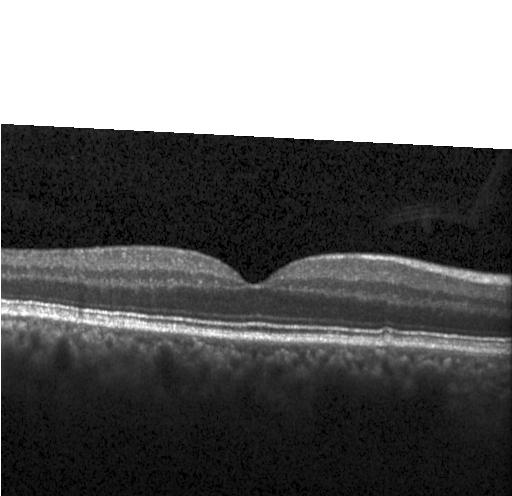
Spectral-domain optical coherence tomography · through the macula · instrument: Heidelberg Spectralis · optical coherence tomography B-scan
Assessment: no evidence of CNV, DME, or drusen.